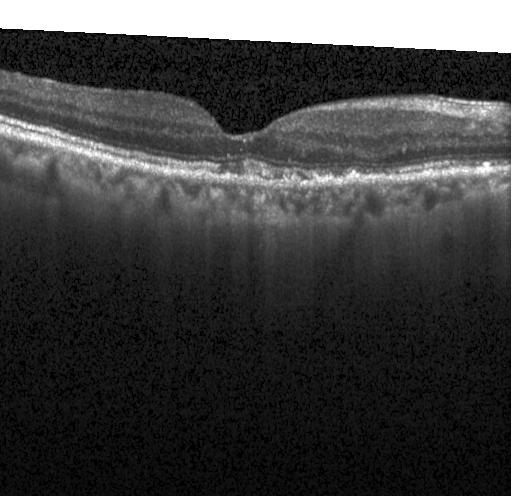 Heidelberg Spectralis; retinal OCT B-scan — The scan shows a choroidal neovascular membrane.